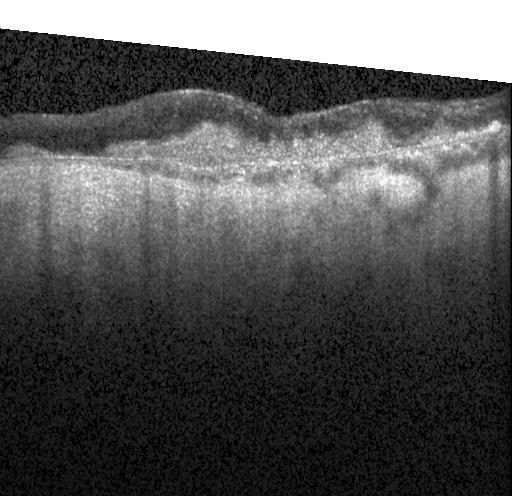 Macular scan · spectral-domain optical coherence tomography · retinal OCT cross-section · Heidelberg Spectralis OCT system — OCT finding: a choroidal neovascular membrane.